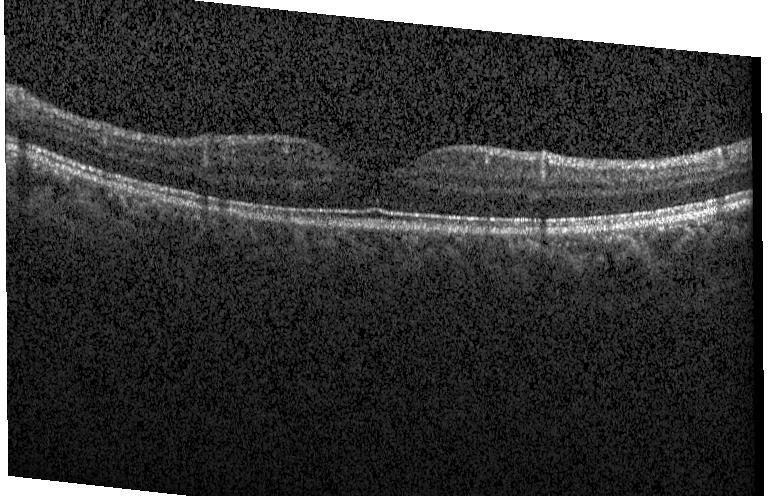
Spectral-domain OCT. Horizontal scan through the fovea. Retinal OCT B-scan.
Finding: no evidence of CNV, DME, or drusen.